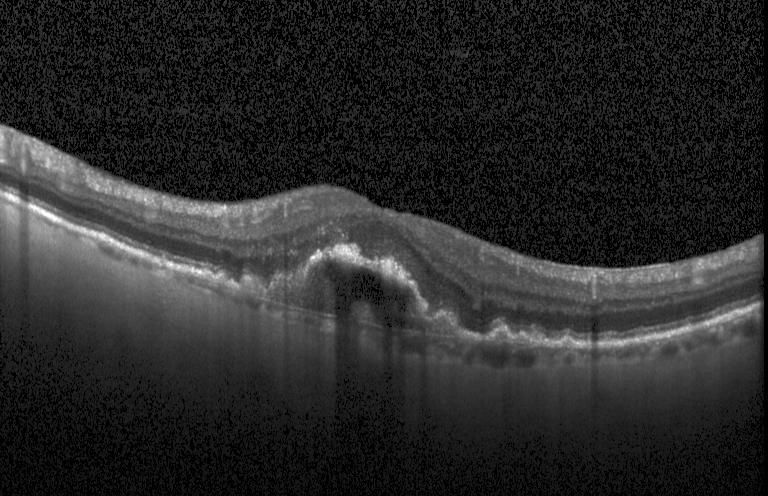 Spectral-domain optical coherence tomography. Macular scan. Heidelberg Spectralis. Optical coherence tomography B-scan.
Dx: choroidal neovascularization (CNV).